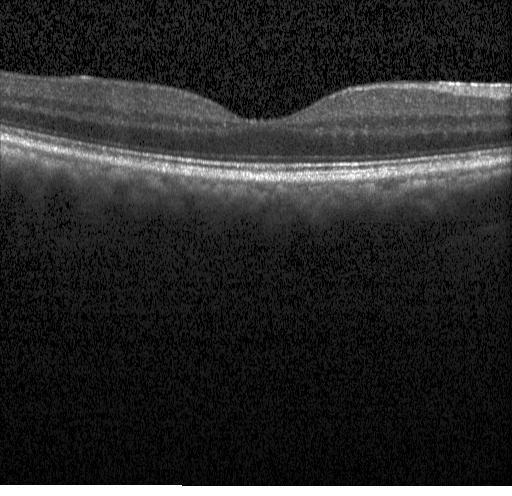

This B-scan demonstrates no evidence of choroidal neovascularization, diabetic macular edema, or drusen.